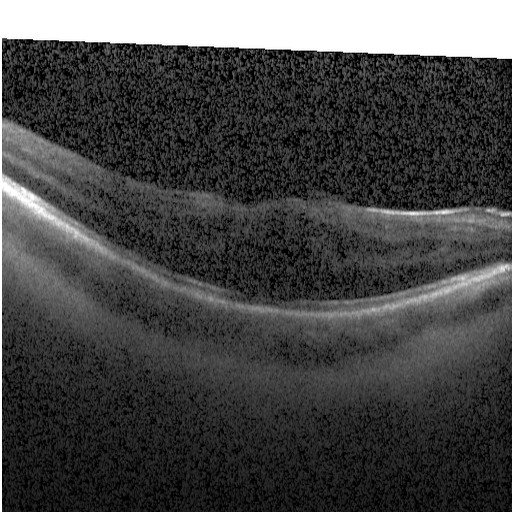

Assessment: diabetic macular edema.